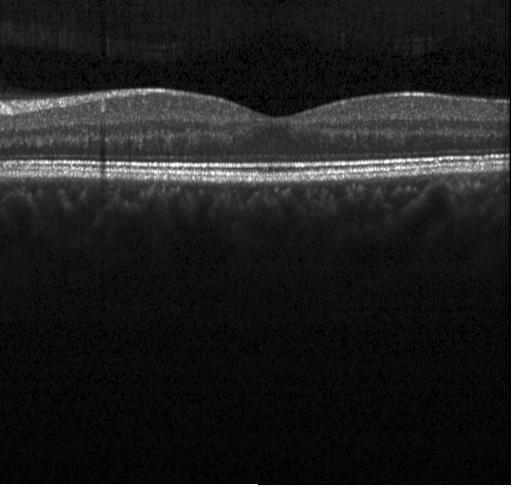

Macular scan; SD-OCT; acquired on a Heidelberg Spectralis; optical coherence tomography B-scan
This B-scan demonstrates neither CNV, DME, nor drusen.